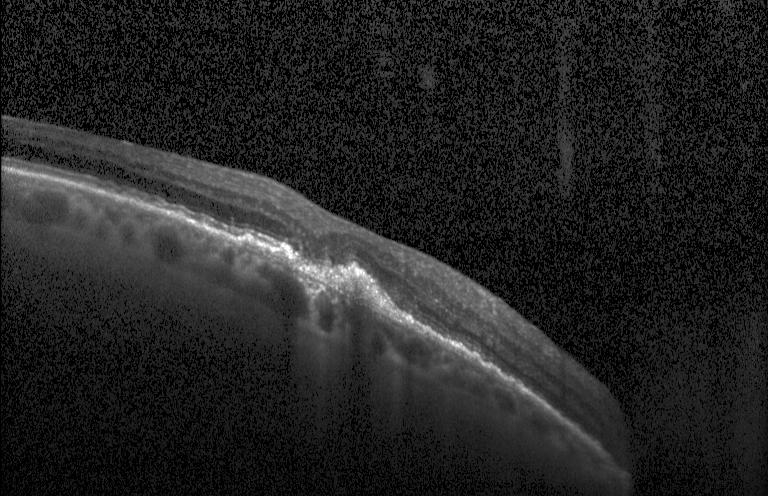

OCT B-scan; spectral-domain OCT — Finding: CNV.